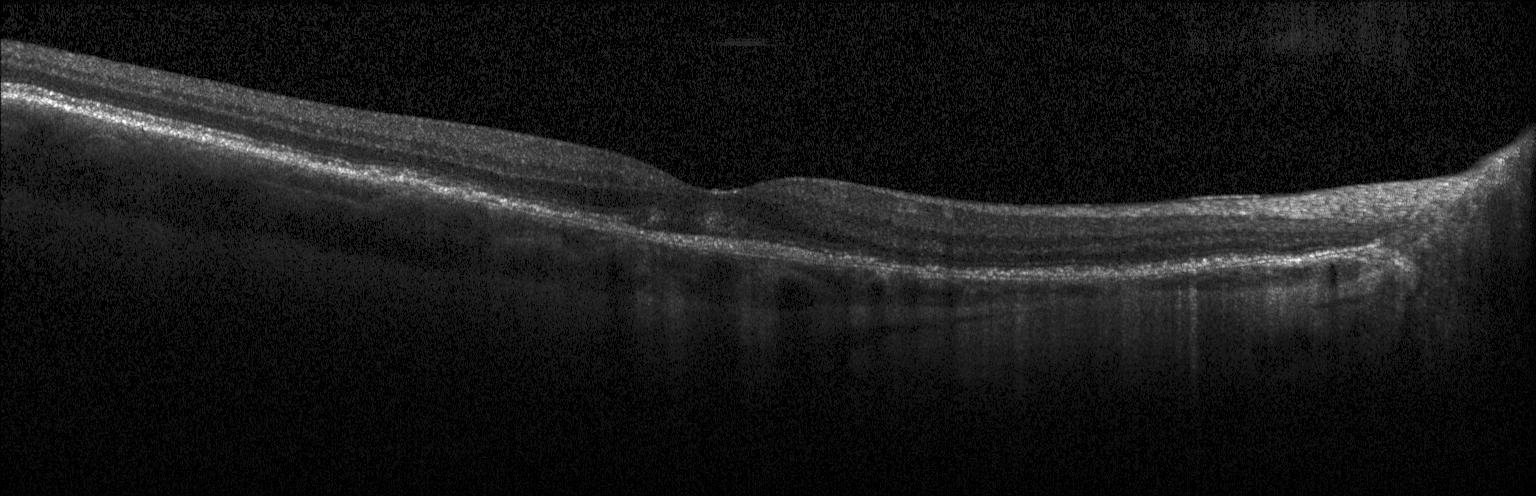
Spectral-domain OCT, OCT line scan, Heidelberg Spectralis.
Assessment: choroidal neovascularization (CNV).